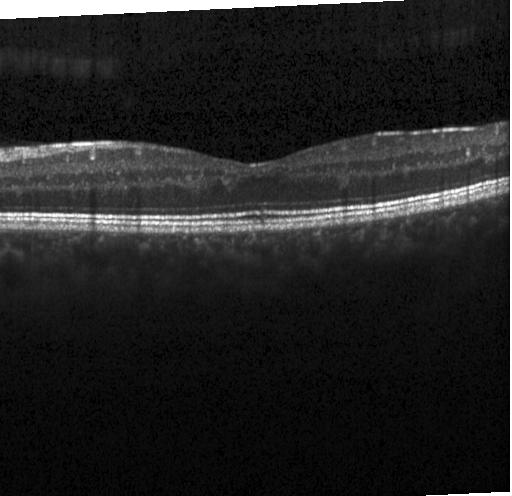 OCT B-scan; SD-OCT; macular scan; instrument: Heidelberg Spectralis — The scan shows no CNV, DME, or drusen.